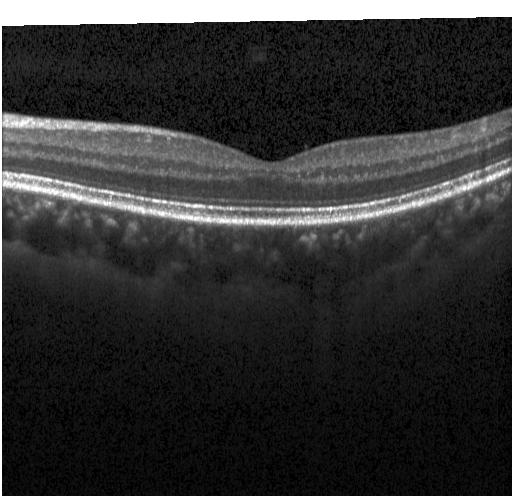
Heidelberg Spectralis OCT system, retinal OCT B-scan, spectral-domain OCT, fovea-centered. The scan shows no choroidal neovascularization, diabetic macular edema, or drusen.